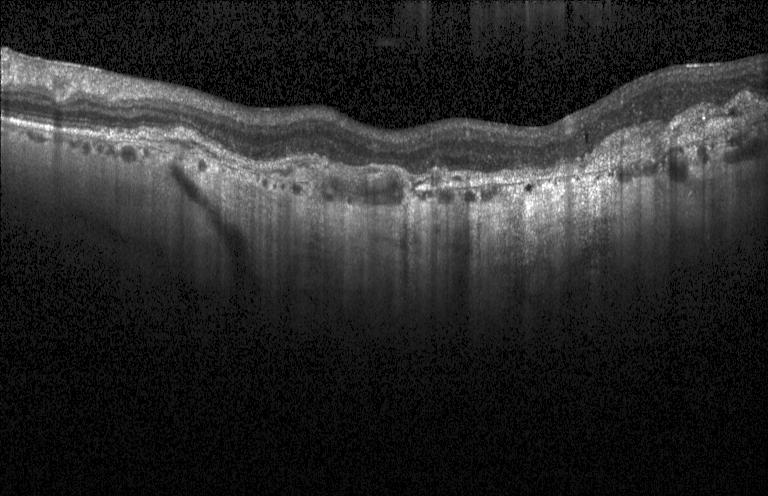
Retinal OCT B-scan. Through the macula — This B-scan demonstrates a choroidal neovascular membrane.